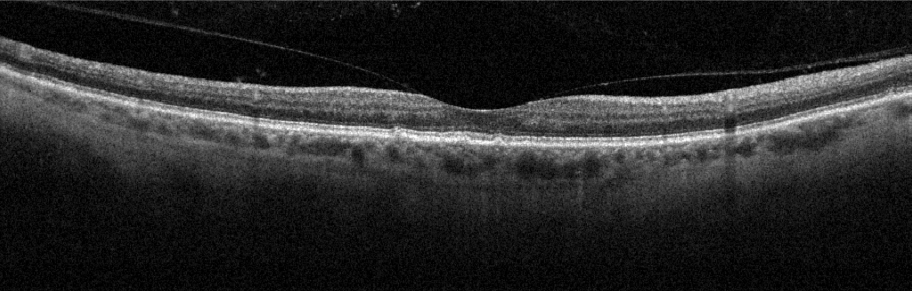
Impression: AMD.